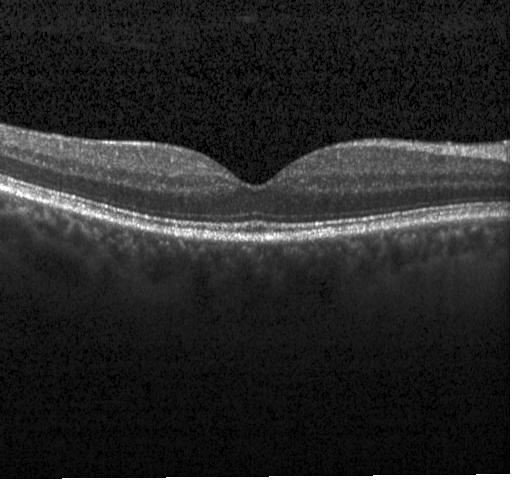

OCT line scan.
No choroidal neovascularization, no diabetic macular edema, and no drusen.